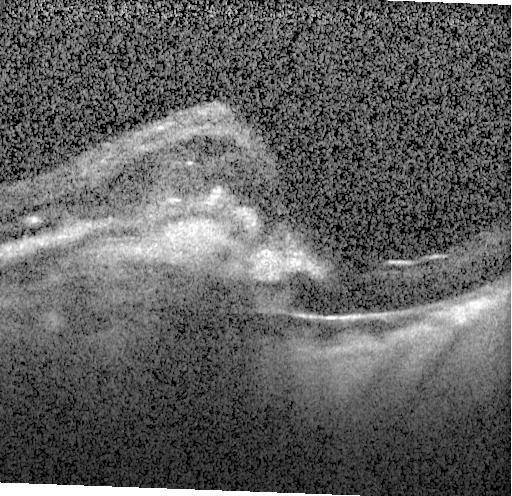 Optical coherence tomography B-scan. Heidelberg Spectralis. Through the macula. Spectral-domain OCT.
Assessment: choroidal neovascularization.